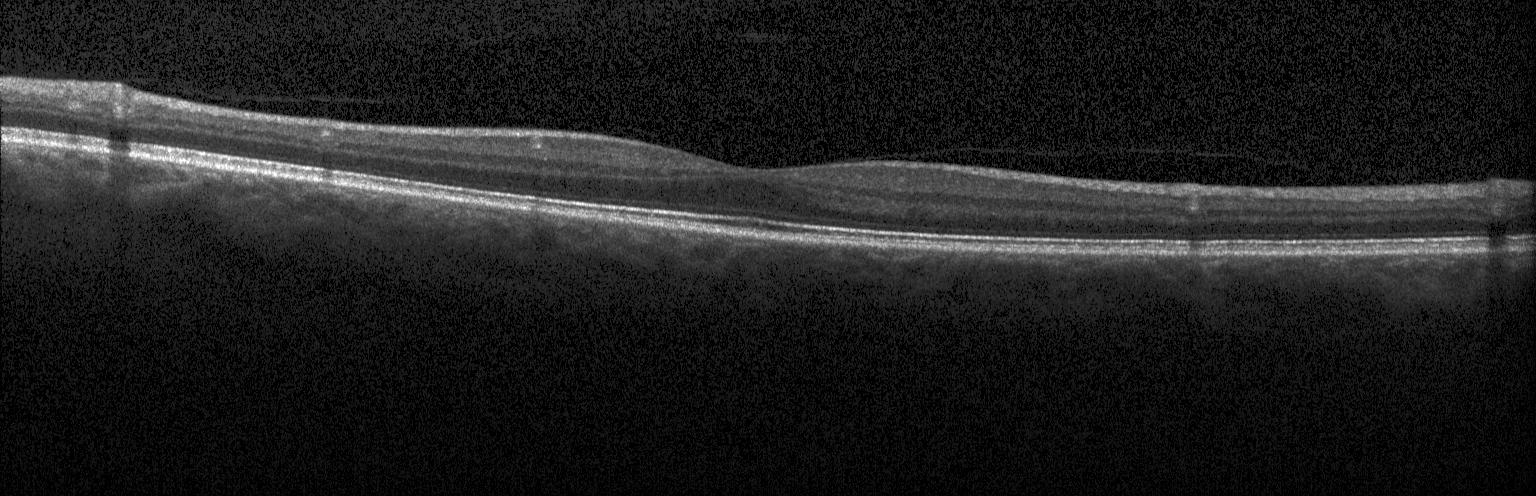

Acquired on a Heidelberg Spectralis, OCT line scan.
Assessment: no evidence of choroidal neovascularization, diabetic macular edema, or drusen.